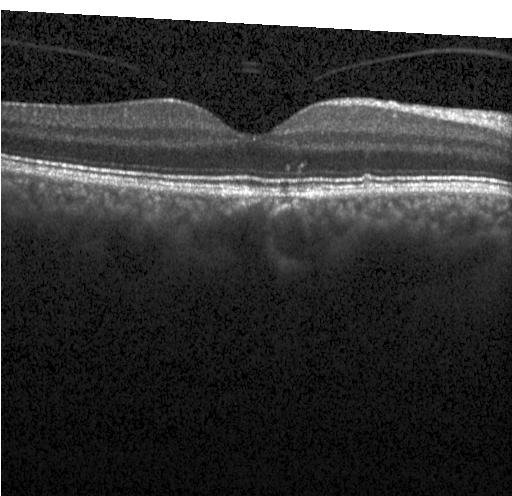

Retinal OCT cross-section showing sub-RPE drusenoid deposits.